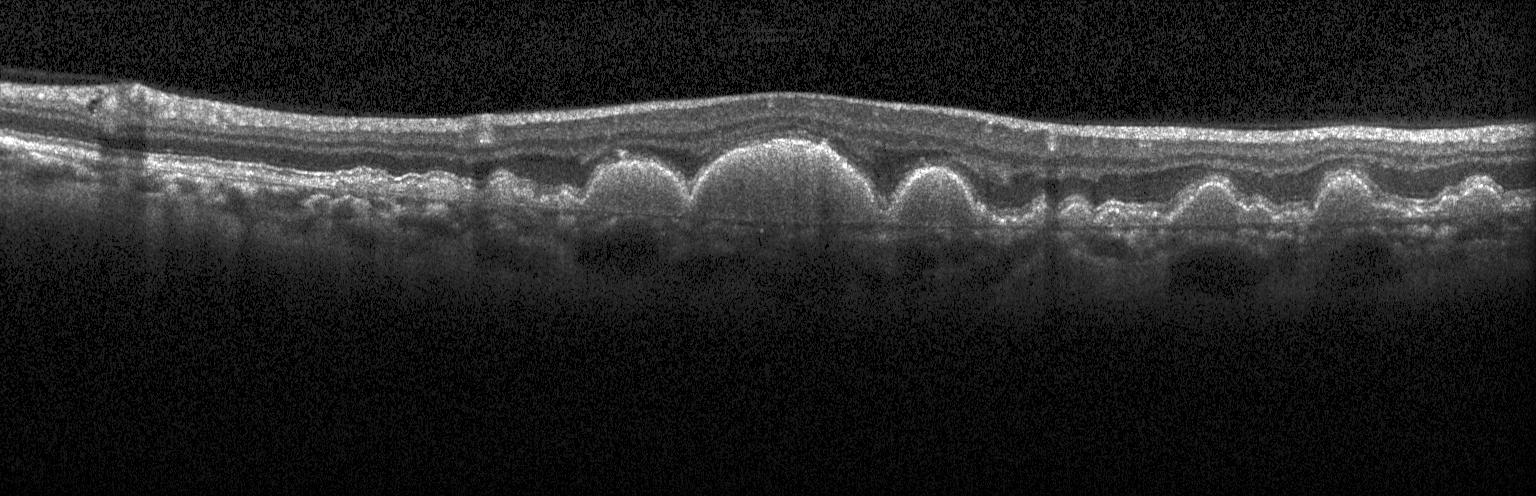
Spectral-domain optical coherence tomography. Macular scan. OCT line scan — Impression: sub-RPE drusenoid deposits.